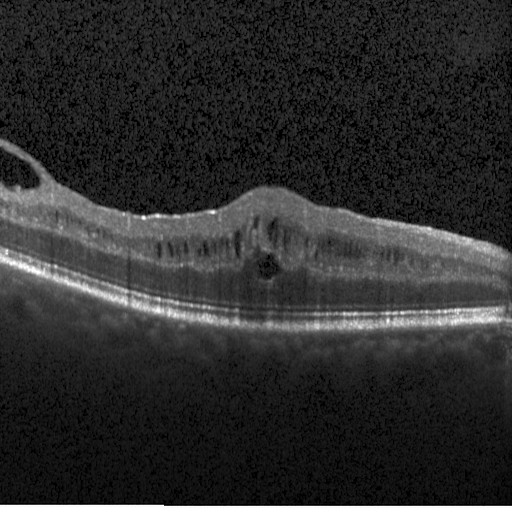 OCT finding: diabetic macular edema (DME).